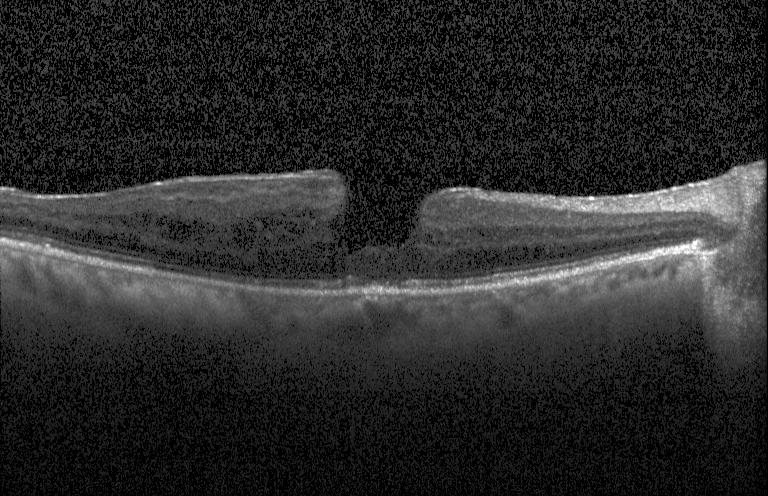 SD-OCT, horizontal scan through the fovea, Heidelberg Spectralis OCT system, optical coherence tomography B-scan.
Impression: diabetic macular edema.